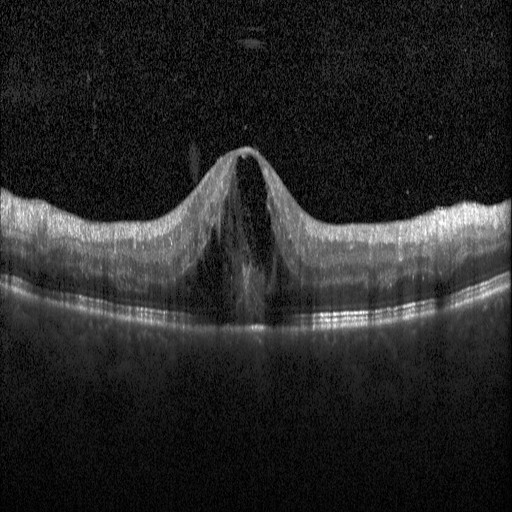
Macular OCT: diabetic macular edema (DME).